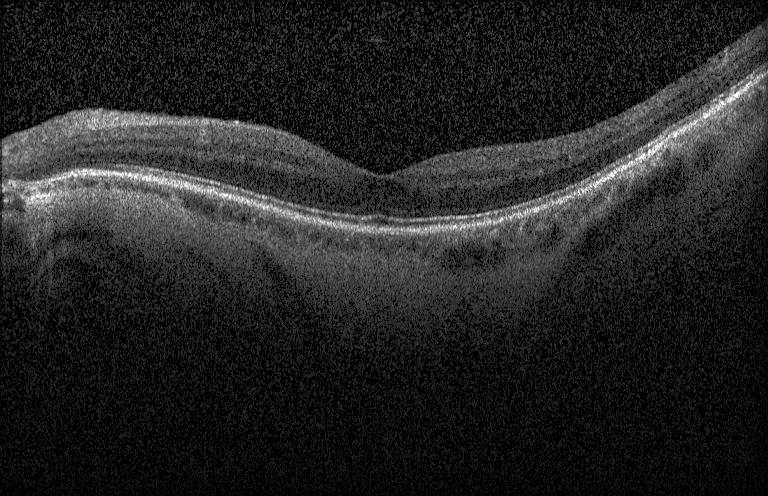 OCT scan showing no choroidal neovascularization, diabetic macular edema, or drusen.